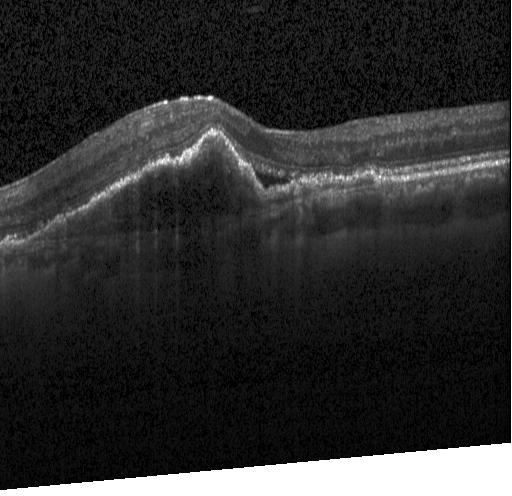

Dx: a choroidal neovascular membrane.